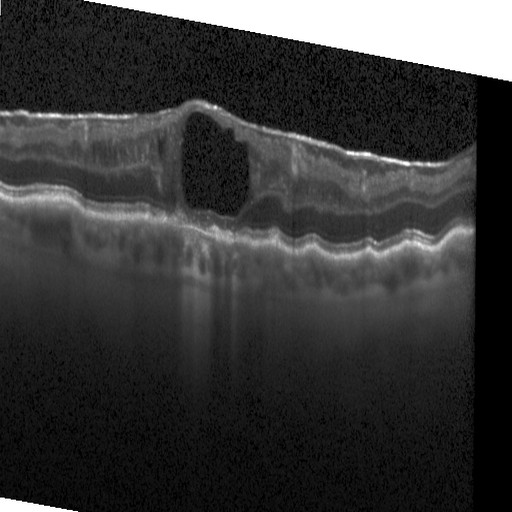
Macular OCT demonstrating DME.